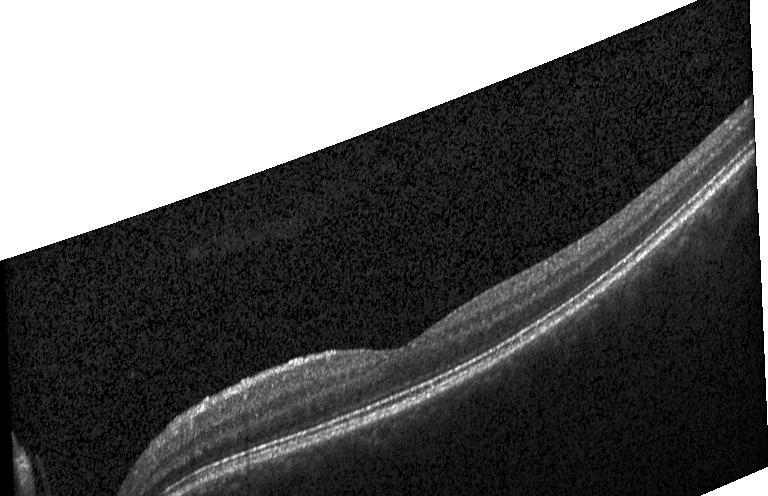 Macular OCT demonstrating no choroidal neovascularization, diabetic macular edema, or drusen.